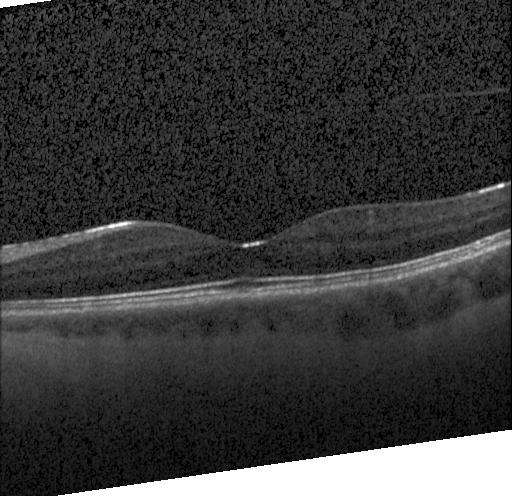

OCT line scan — No evidence of choroidal neovascularization, diabetic macular edema, or drusen.